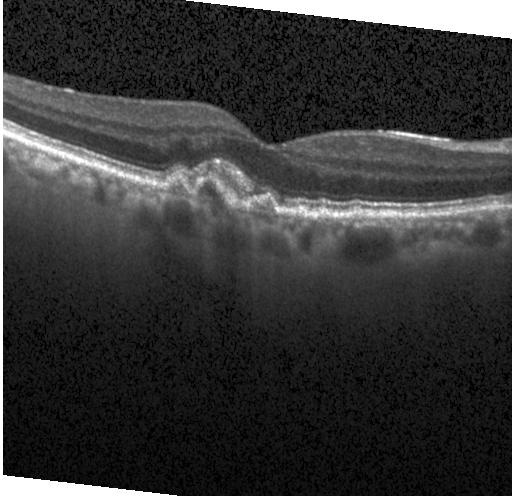
Retinal OCT B-scan — Impression: a choroidal neovascular membrane.